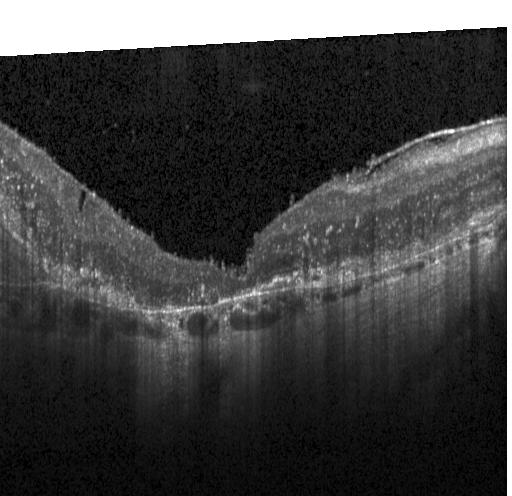
Impression: choroidal neovascularization.